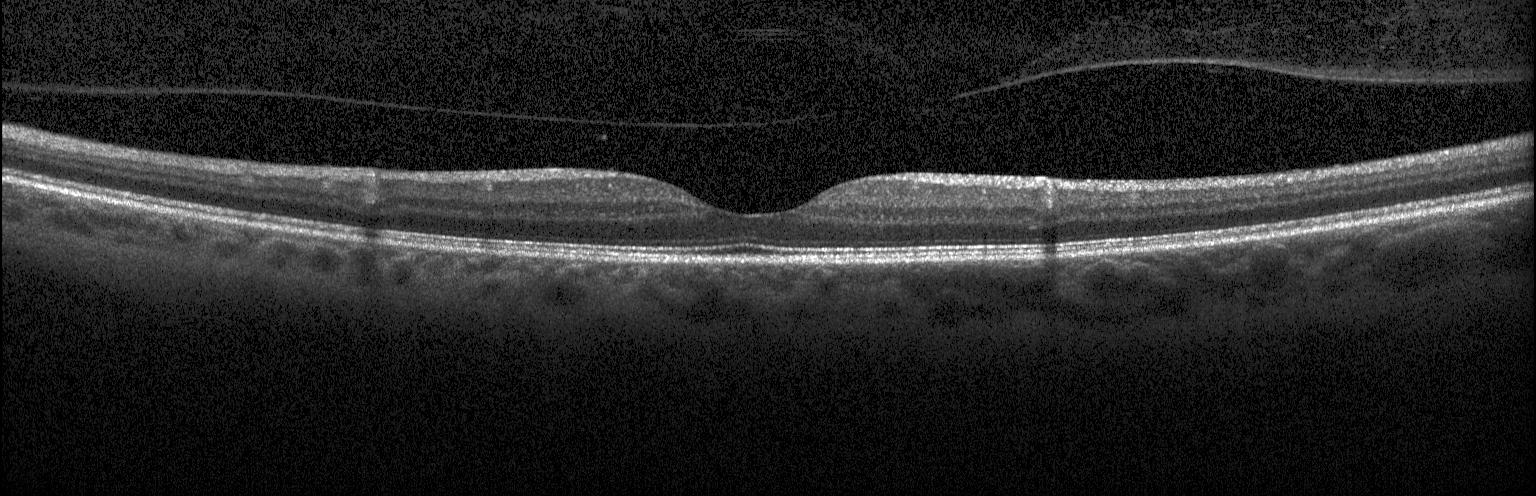 Heidelberg Spectralis OCT system · optical coherence tomography B-scan · macular scan · spectral-domain OCT
Finding: no evidence of choroidal neovascularization, diabetic macular edema, or drusen.